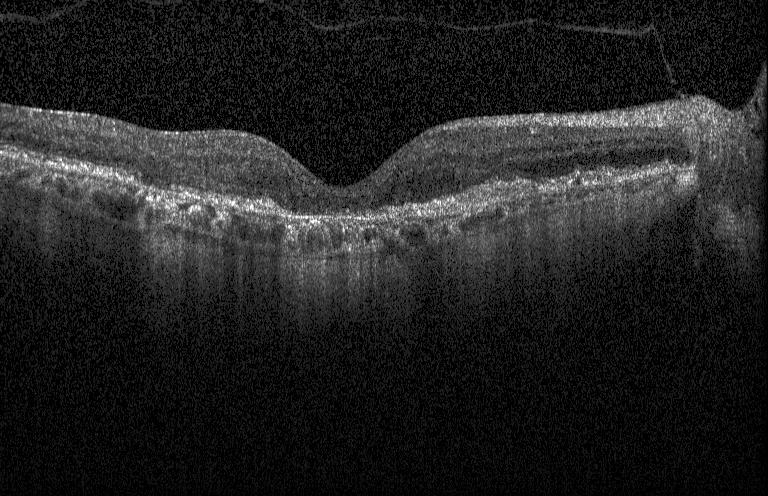 OCT finding: a choroidal neovascular membrane.